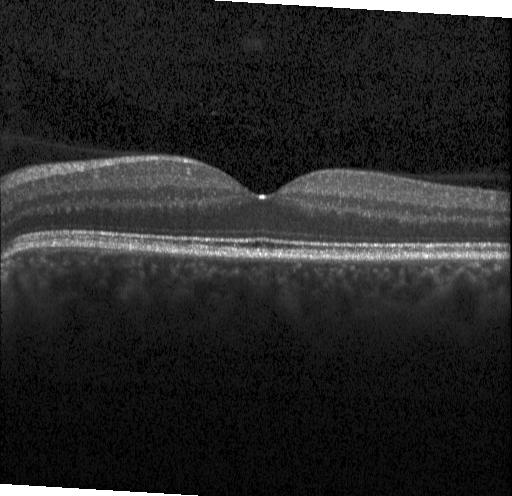
Retinal OCT B-scan · through the macula · acquired on a Heidelberg Spectralis · SD-OCT
OCT finding: no evidence of choroidal neovascularization, diabetic macular edema, or drusen.